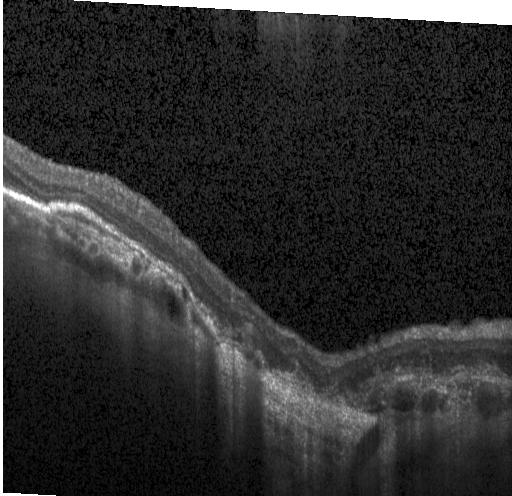 Optical coherence tomography B-scan. Centered on the fovea. Dx: CNV.